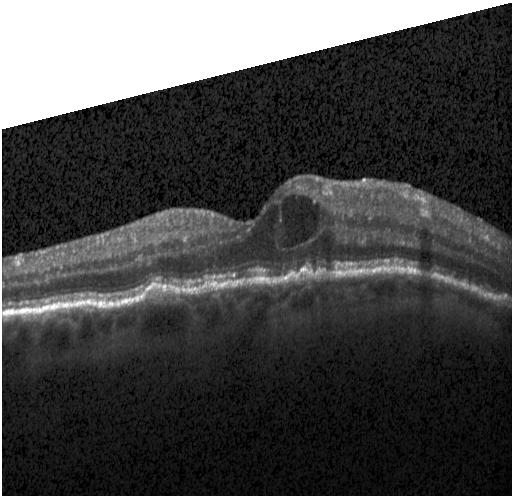 Impression: a choroidal neovascular membrane.